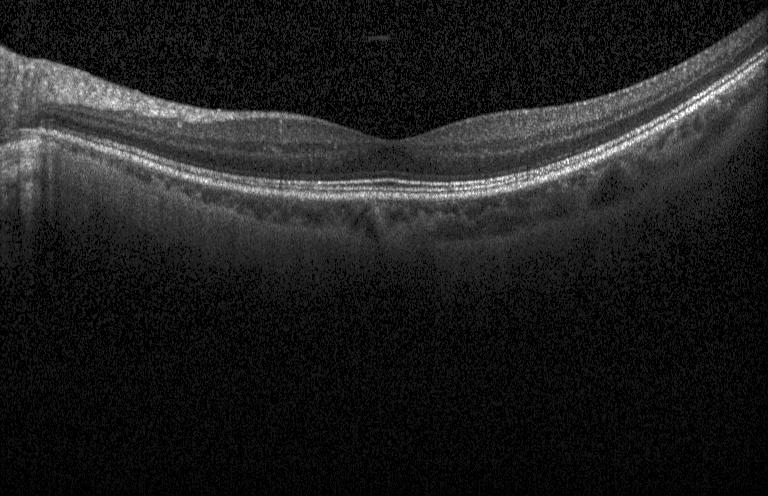

Spectral-domain OCT; optical coherence tomography scan.
Assessment: no choroidal neovascularization, diabetic macular edema, or drusen.